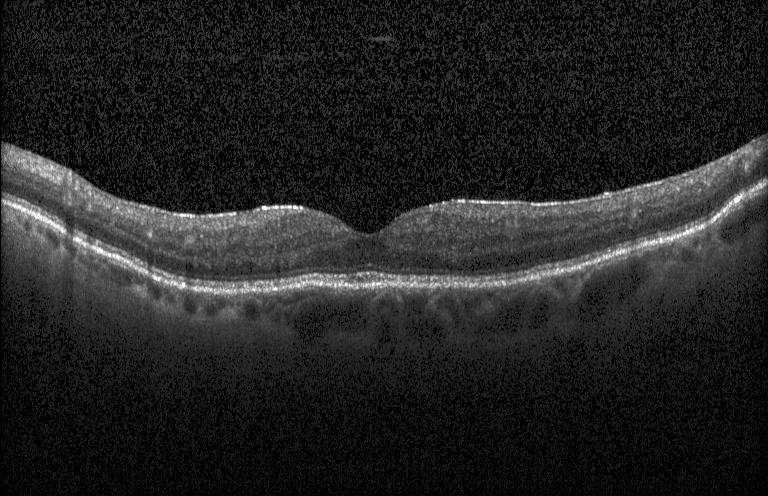 SD-OCT. OCT line scan — OCT finding: neither choroidal neovascularization, diabetic macular edema, nor drusen.